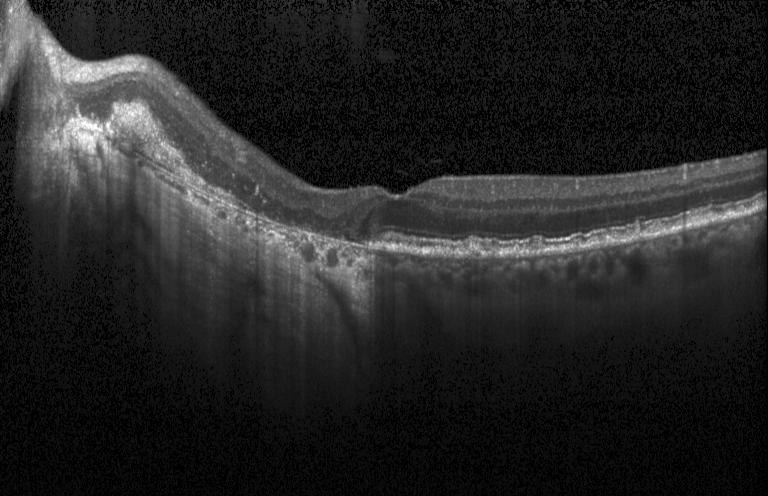

Macular OCT: a choroidal neovascular membrane.